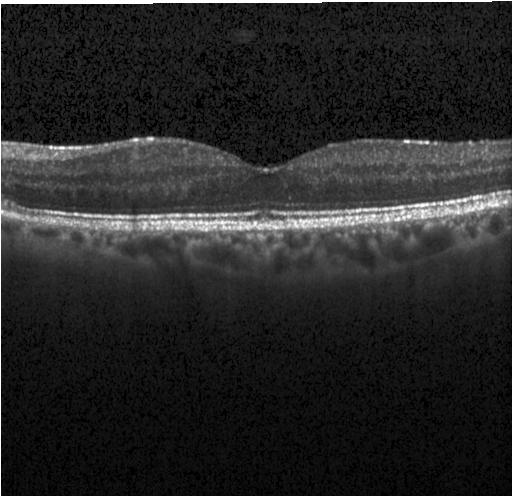
Optical coherence tomography scan.
The scan shows neither choroidal neovascularization, diabetic macular edema, nor drusen.